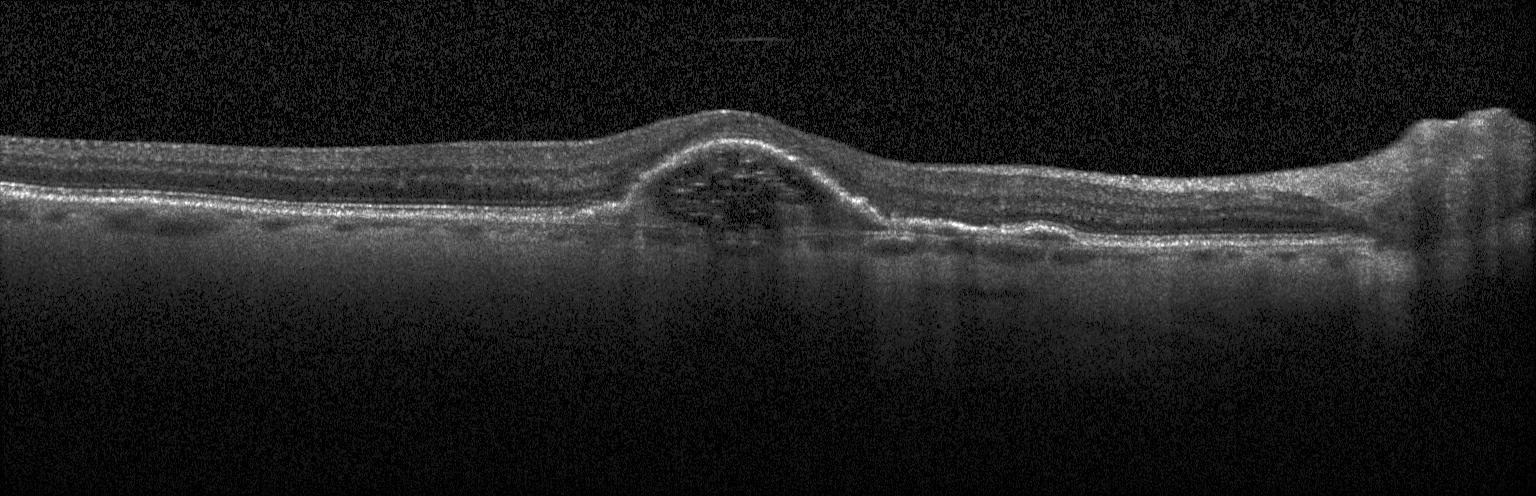 The scan shows a choroidal neovascular membrane.